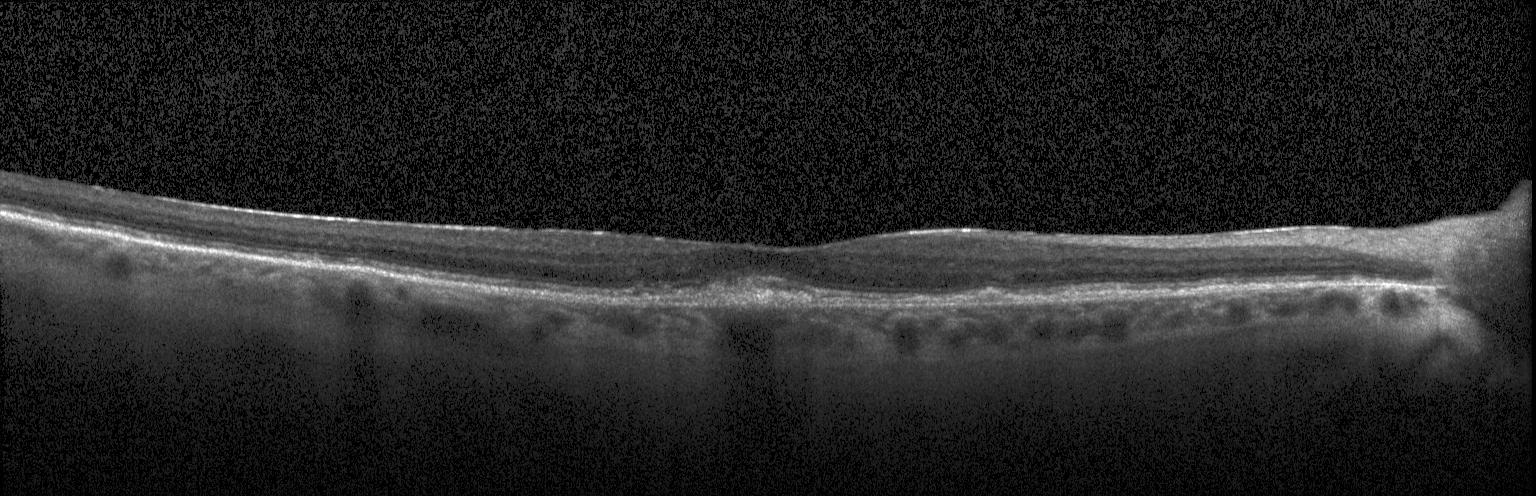
Spectral-domain OCT; OCT line scan
Finding: a choroidal neovascular membrane.